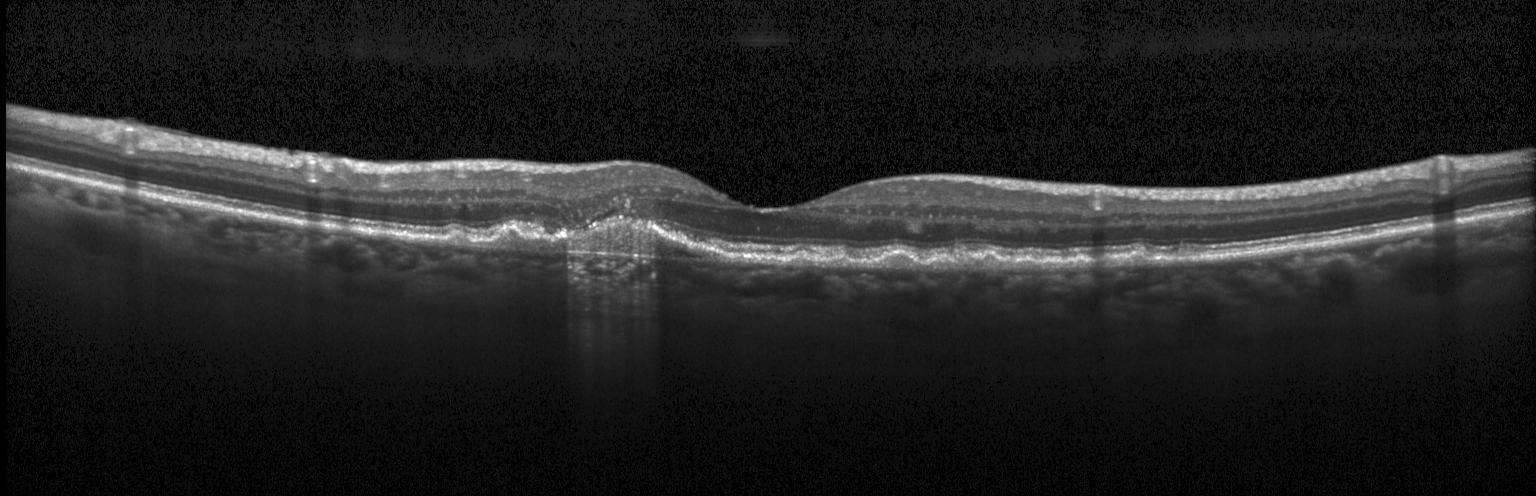

Optical coherence tomography scan; Heidelberg Spectralis
Assessment: choroidal neovascularization (CNV).